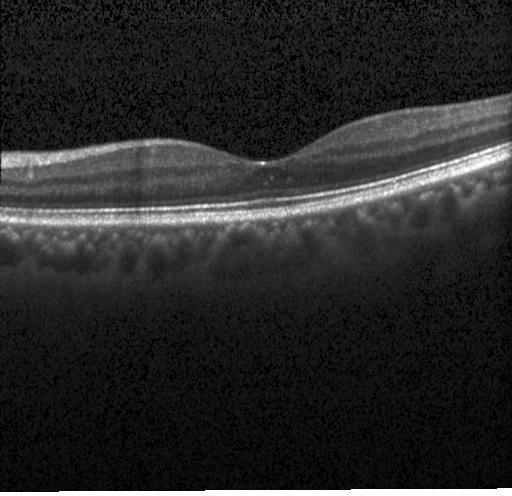 Retinal OCT B-scan. No evidence of choroidal neovascularization, diabetic macular edema, or drusen.